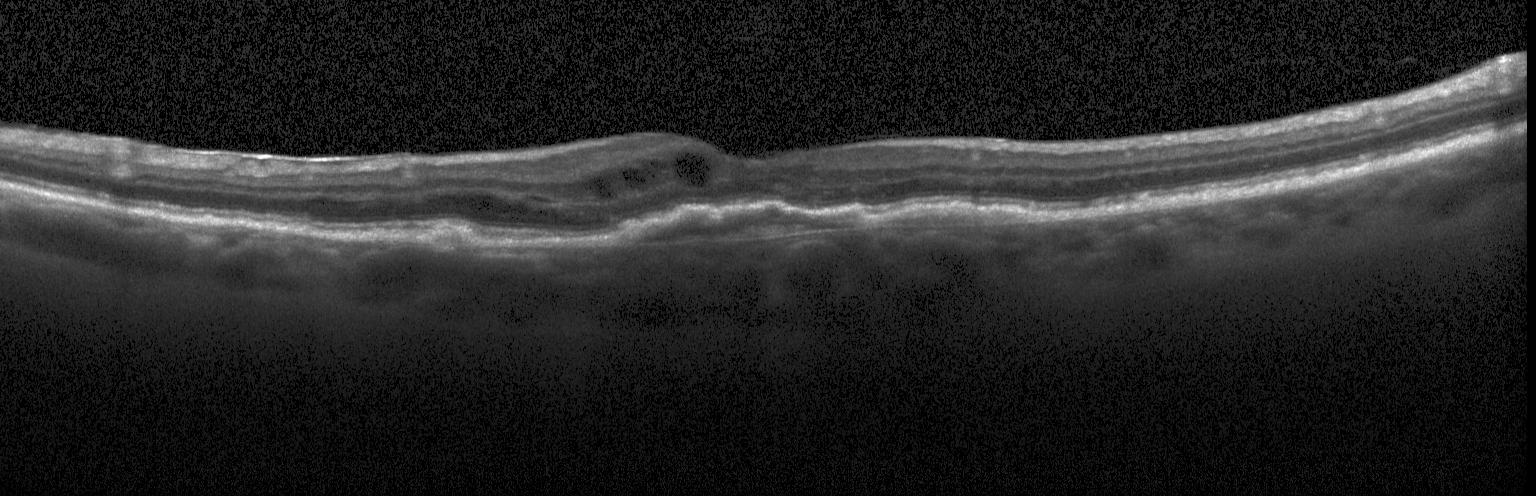 Spectral-domain optical coherence tomography; optical coherence tomography B-scan; fovea-centered; instrument: Heidelberg Spectralis.
Diagnosis: choroidal neovascularization (CNV).